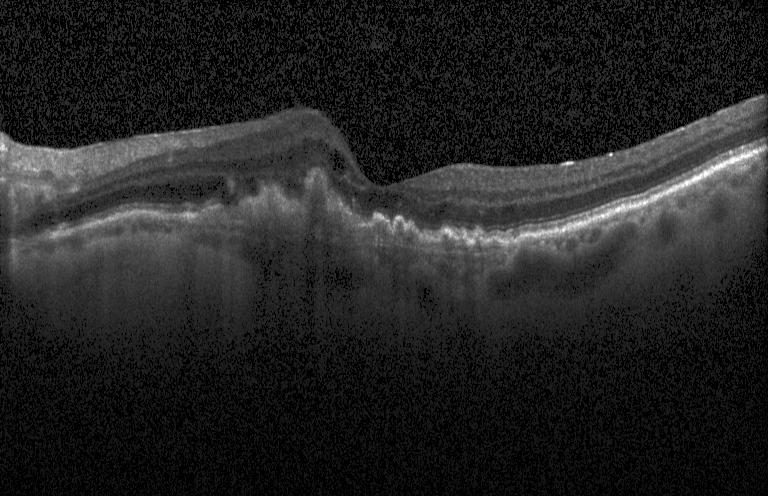 Fovea-centered; retinal OCT B-scan
Diagnosis: a choroidal neovascular membrane.